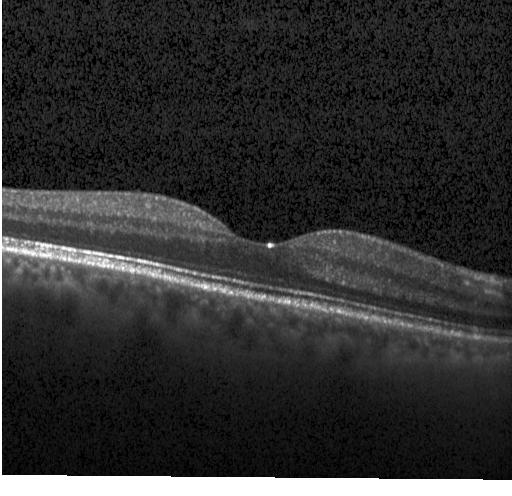

OCT line scan, spectral-domain optical coherence tomography — Assessment: no evidence of choroidal neovascularization, diabetic macular edema, or drusen.